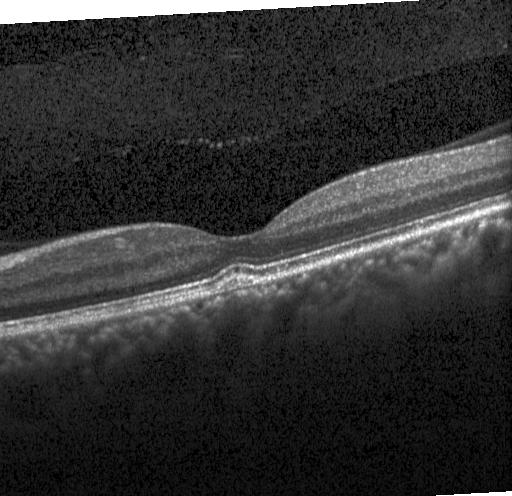

Spectral-domain OCT. Optical coherence tomography scan — The scan shows sub-RPE drusenoid deposits.